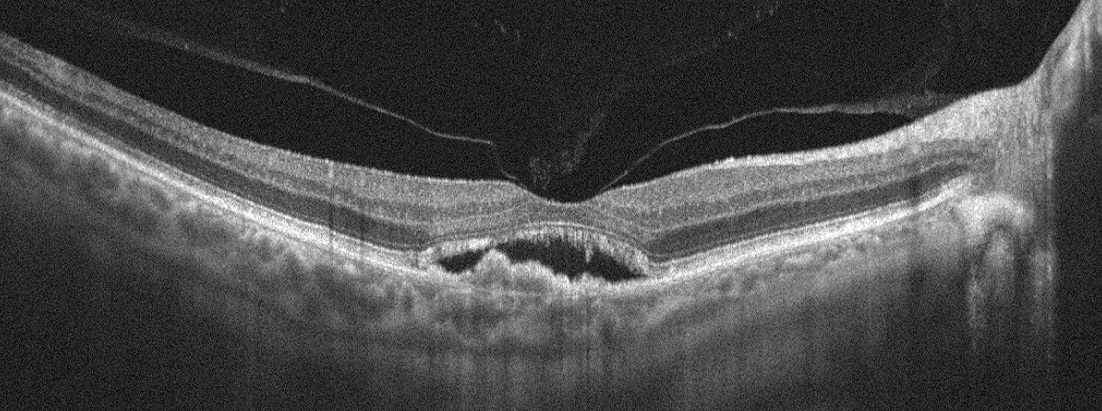

Optical coherence tomography scan. This B-scan demonstrates age-related macular degeneration.